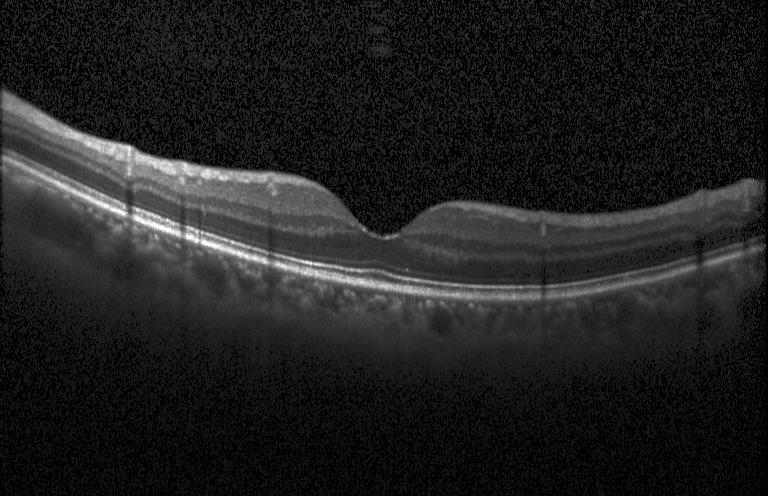 Heidelberg Spectralis; spectral-domain optical coherence tomography; OCT line scan; fovea-centered.
Assessment: no evidence of choroidal neovascularization, diabetic macular edema, or drusen.